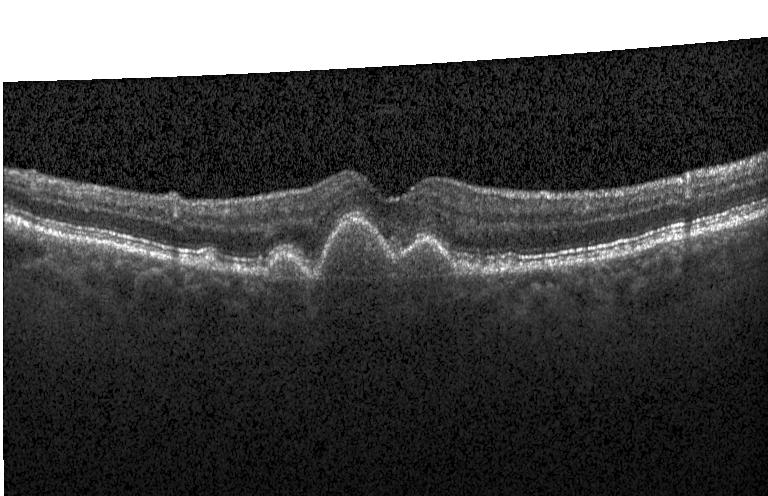 Fovea-centered, Heidelberg Spectralis, SD-OCT, retinal OCT B-scan — This B-scan demonstrates a choroidal neovascular membrane.